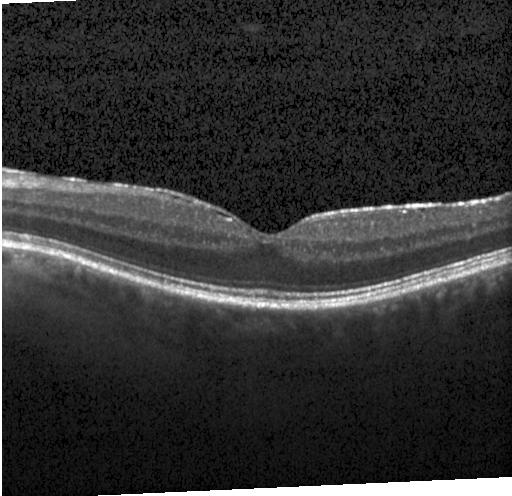 This B-scan demonstrates no choroidal neovascularization, diabetic macular edema, or drusen.